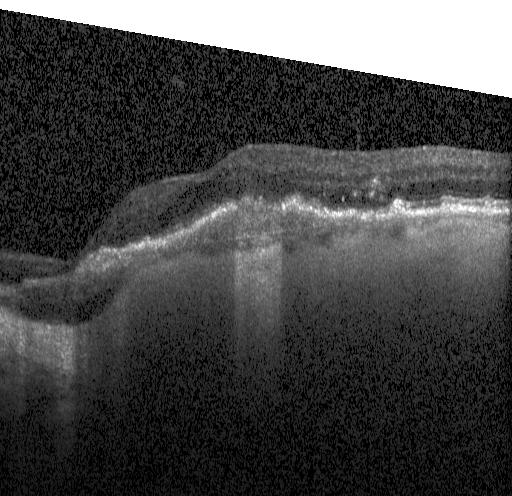
OCT B-scan · through the macula · spectral-domain optical coherence tomography. This B-scan demonstrates a choroidal neovascular membrane.